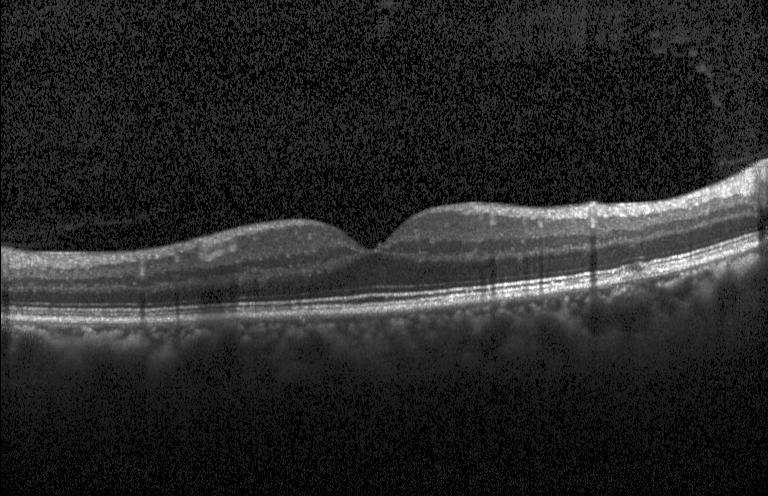

Assessment: no CNV, no DME, and no drusen.